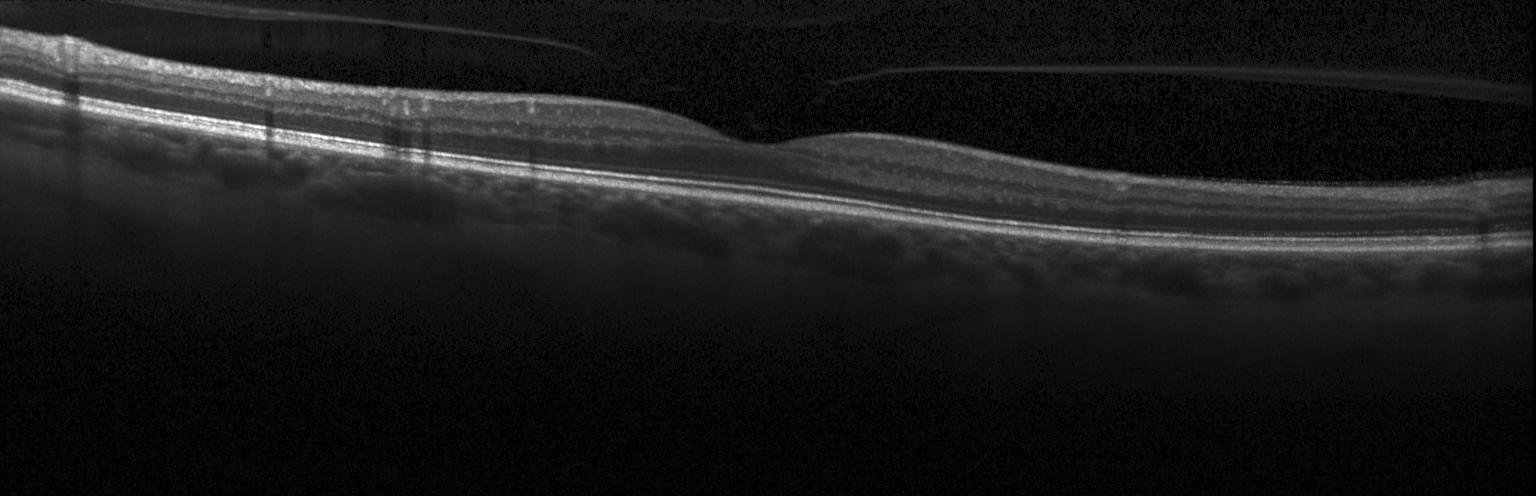 Heidelberg Spectralis · OCT B-scan · centered on the fovea · spectral-domain OCT. This B-scan demonstrates no choroidal neovascularization, no diabetic macular edema, and no drusen.